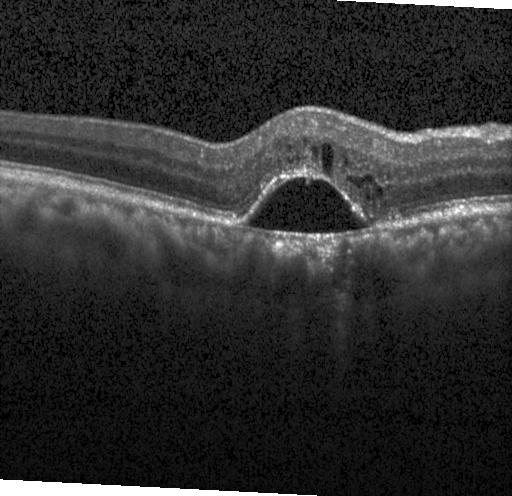 OCT B-scan. Impression: choroidal neovascularization.